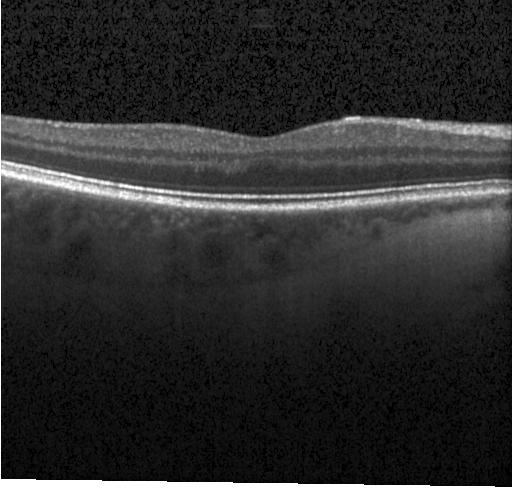
Impression: no choroidal neovascularization, diabetic macular edema, or drusen.